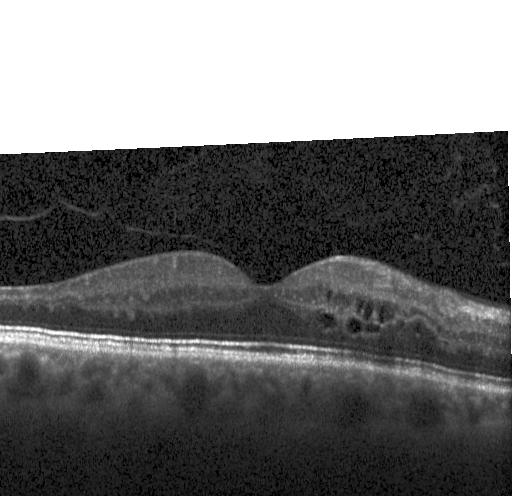 Through the macula. OCT line scan — The scan shows diabetic macular edema (DME).